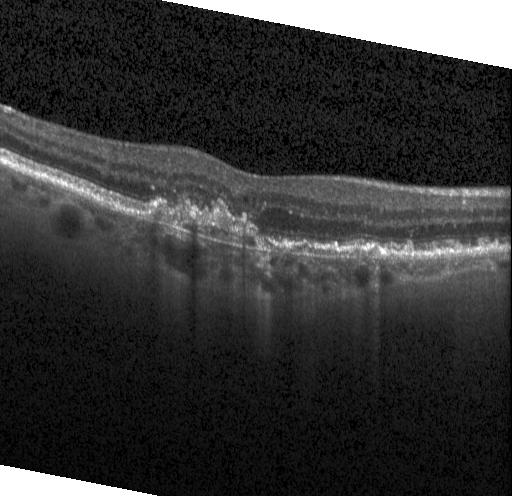

Assessment: a choroidal neovascular membrane.